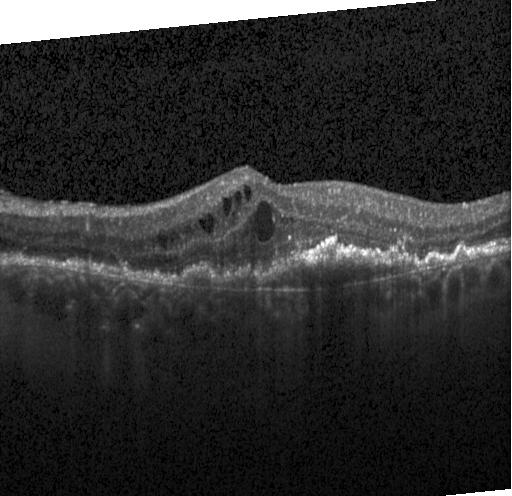 Retinal OCT cross-section
Assessment: CNV.